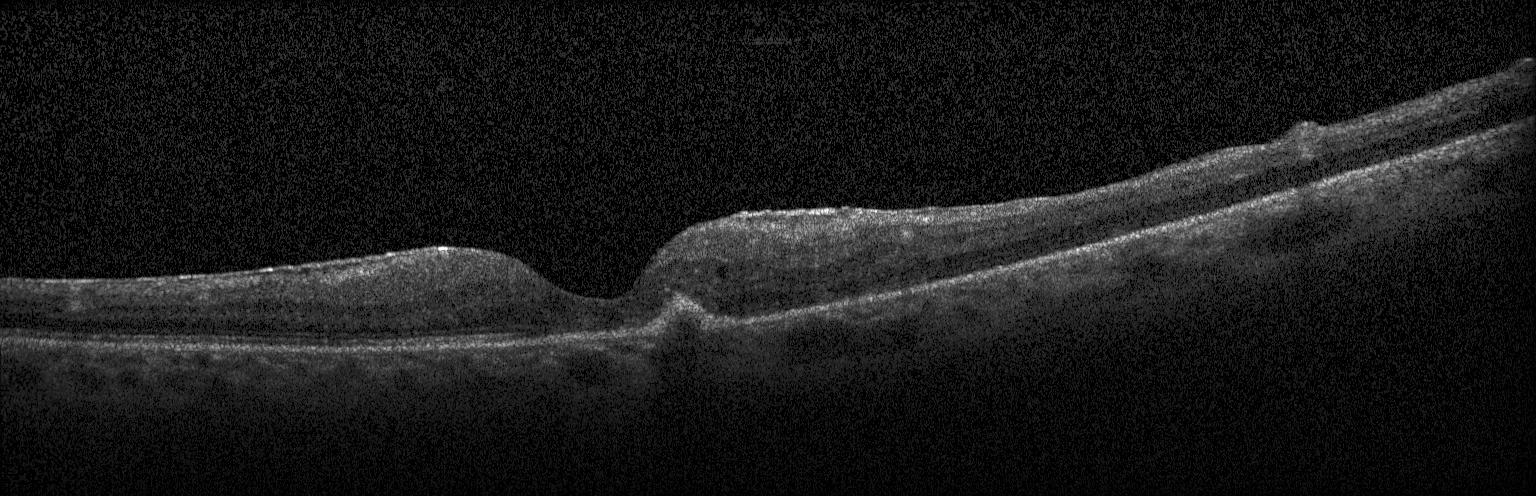 OCT B-scan. Diagnosis: choroidal neovascularization.